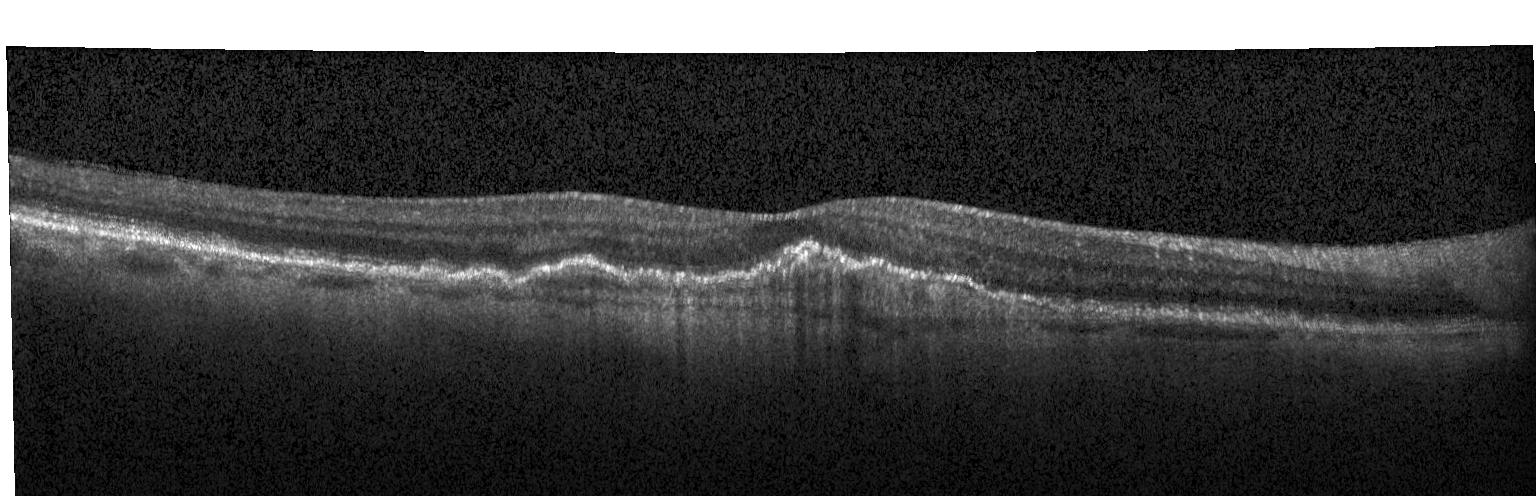
Macular OCT demonstrating a choroidal neovascular membrane.